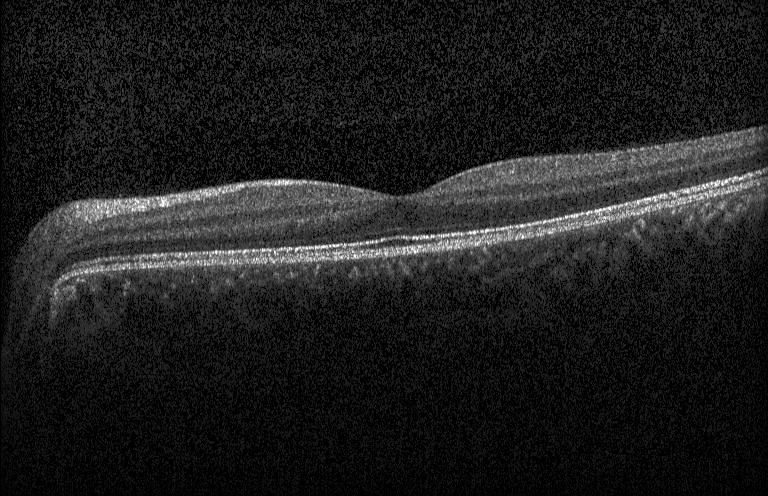 Diagnosis: no choroidal neovascularization, diabetic macular edema, or drusen.